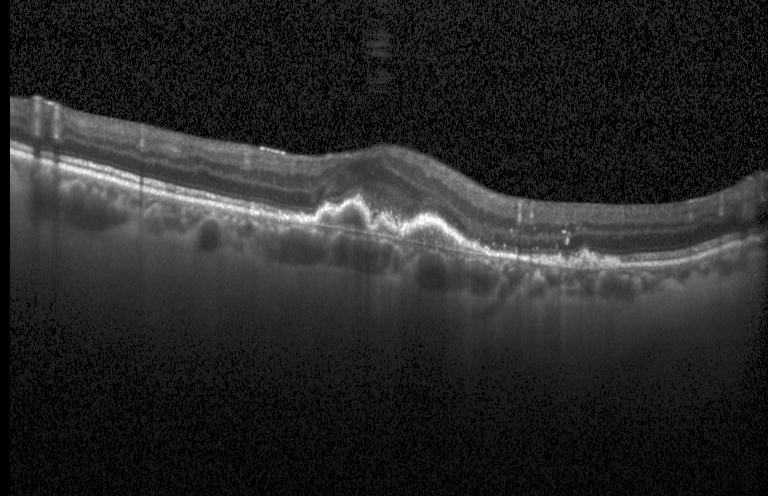
Spectral-domain OCT, OCT line scan. Diagnosis: choroidal neovascularization.